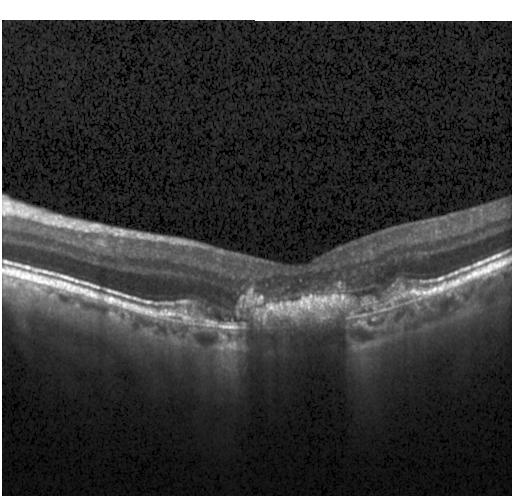 OCT scan showing choroidal neovascularization.